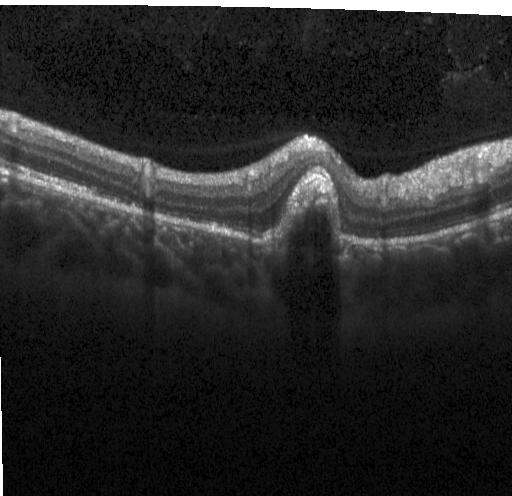
Through the macula. Optical coherence tomography B-scan. SD-OCT. Heidelberg Spectralis — Diagnosis: choroidal neovascularization.